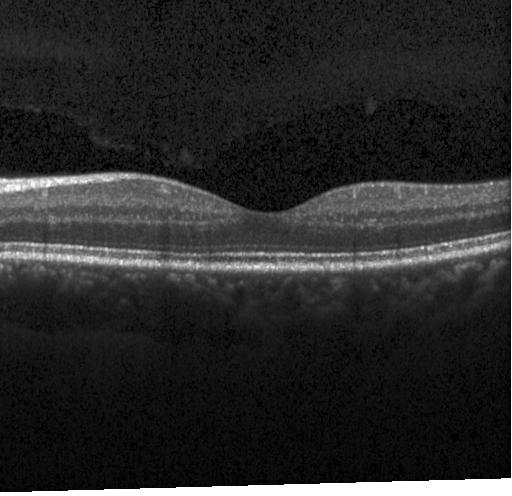

SD-OCT. Heidelberg Spectralis. OCT line scan. Centered on the fovea. The scan shows no choroidal neovascularization, no diabetic macular edema, and no drusen.